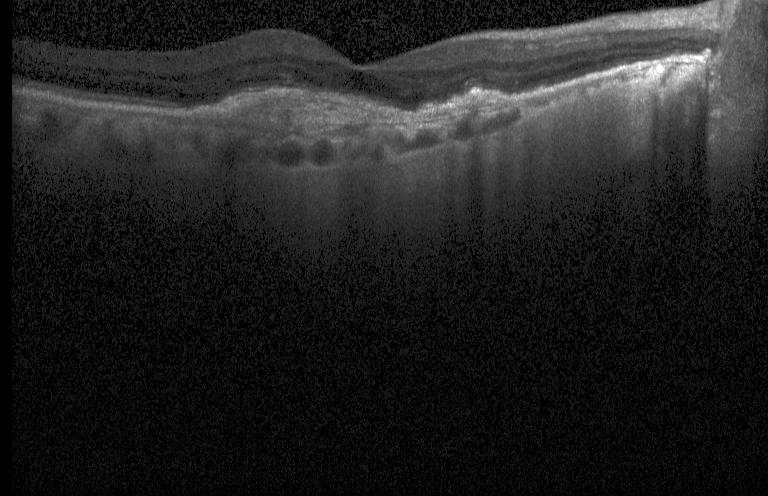

Assessment: choroidal neovascularization.